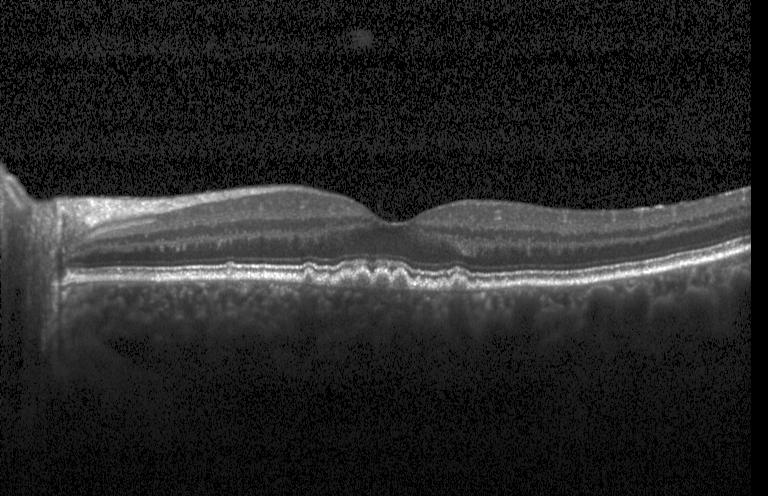

Drusen.